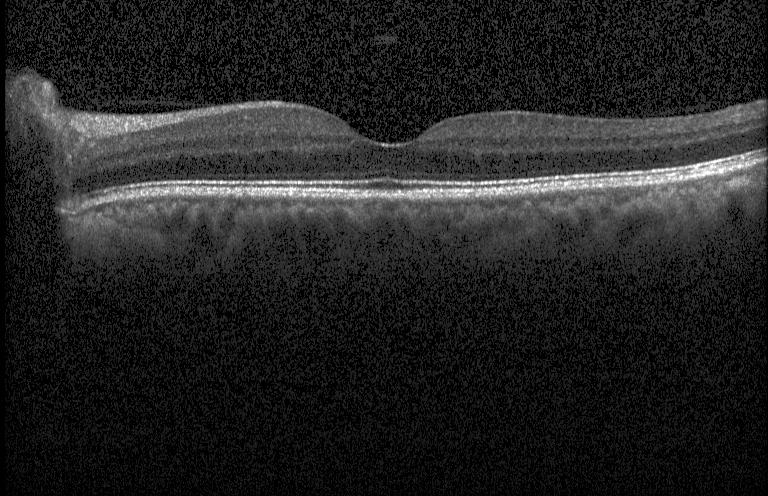
Diagnosis: no choroidal neovascularization, diabetic macular edema, or drusen.